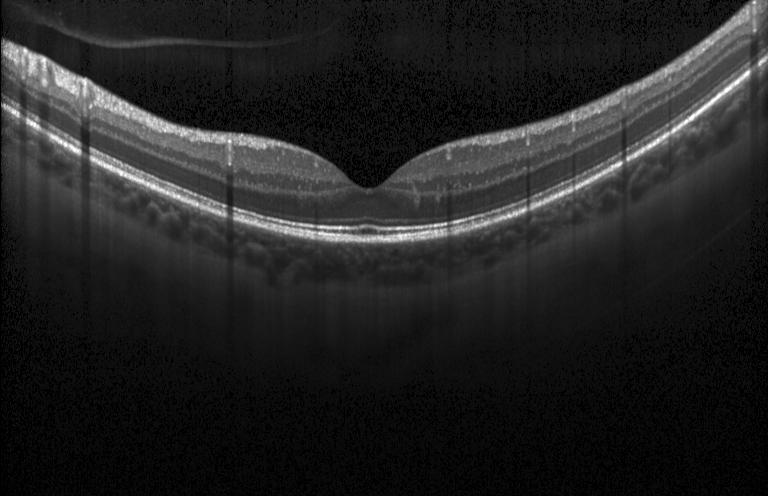
Neither choroidal neovascularization, diabetic macular edema, nor drusen.